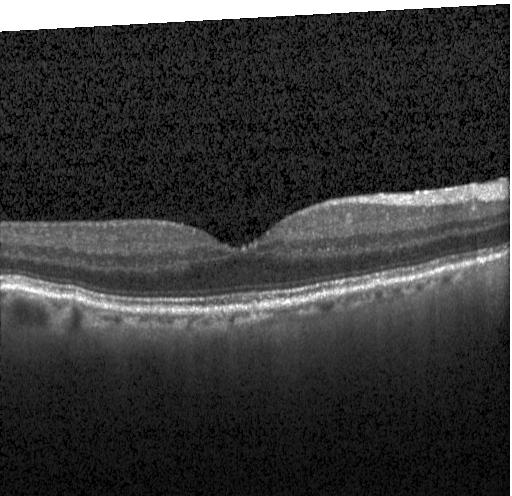

Spectral-domain OCT, centered on the fovea, retinal OCT B-scan, Heidelberg Spectralis OCT system
Finding: no choroidal neovascularization, diabetic macular edema, or drusen.